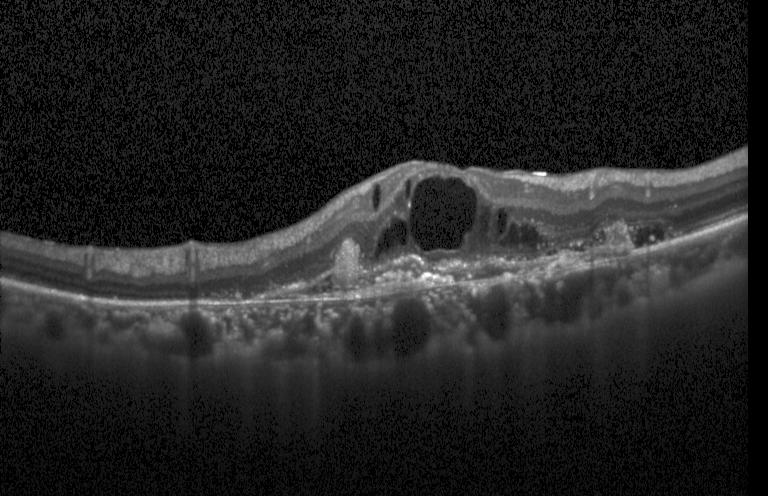 Impression: choroidal neovascularization (CNV).